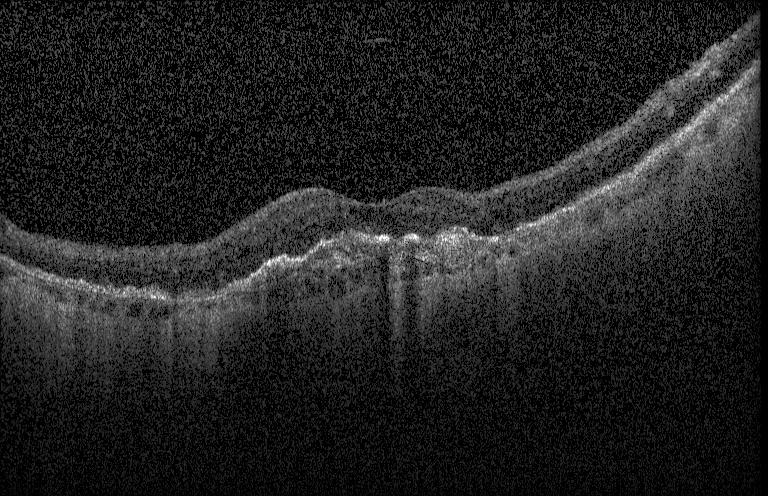 Spectral-domain OCT · retinal OCT cross-section · centered on the fovea · Heidelberg Spectralis — Impression: choroidal neovascularization (CNV).